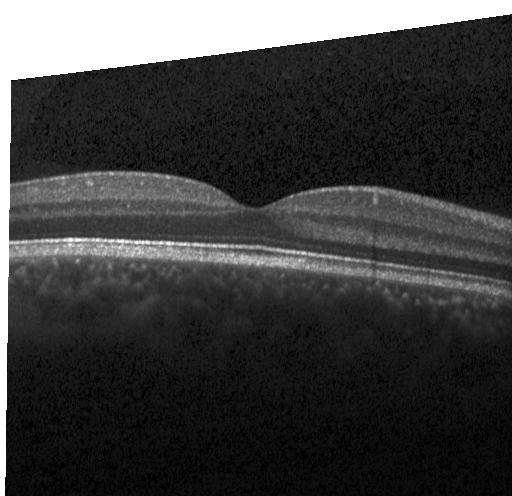

Impression: no choroidal neovascularization, diabetic macular edema, or drusen.